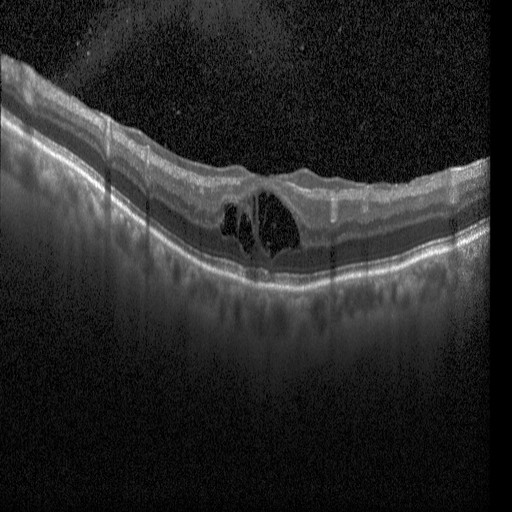
Retinal OCT cross-section
Macular OCT: diabetic macular edema (DME).